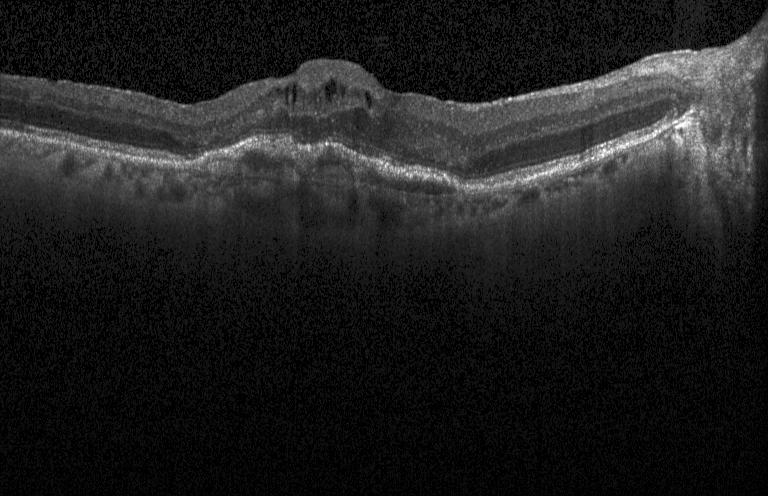 Choroidal neovascularization (CNV).